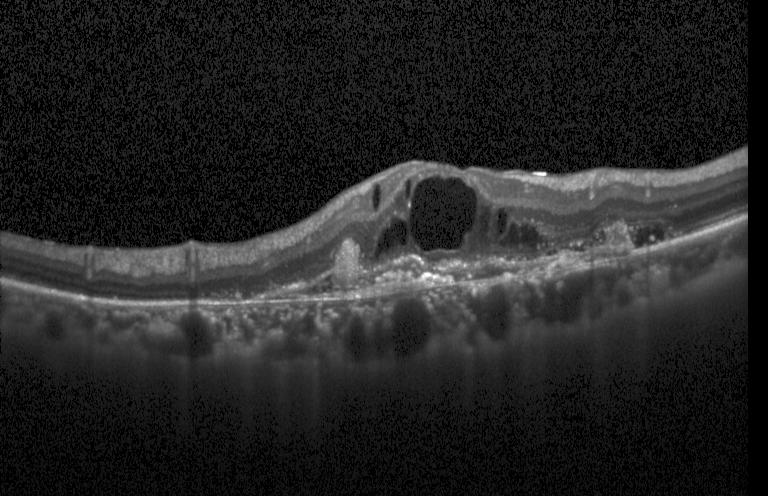
This B-scan demonstrates CNV.